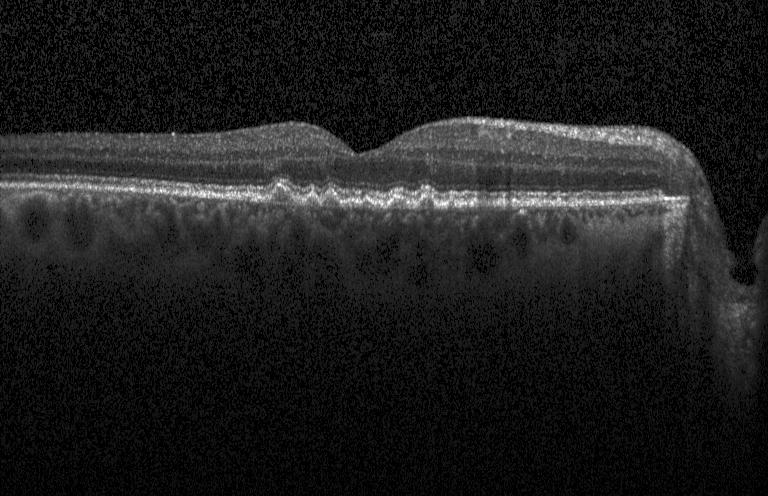 Macular OCT demonstrating sub-RPE drusenoid deposits.